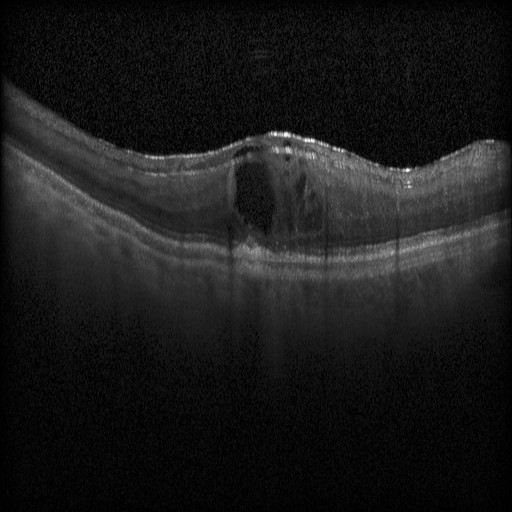 Diagnosis: DME.